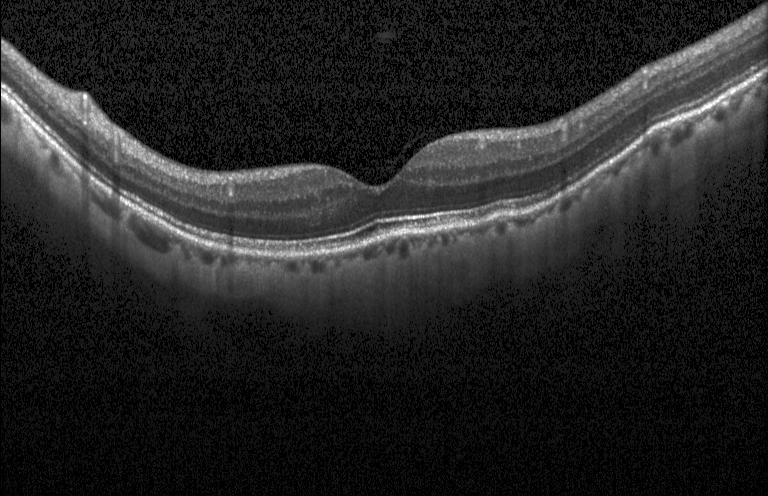
Macular OCT: no choroidal neovascularization, diabetic macular edema, or drusen.